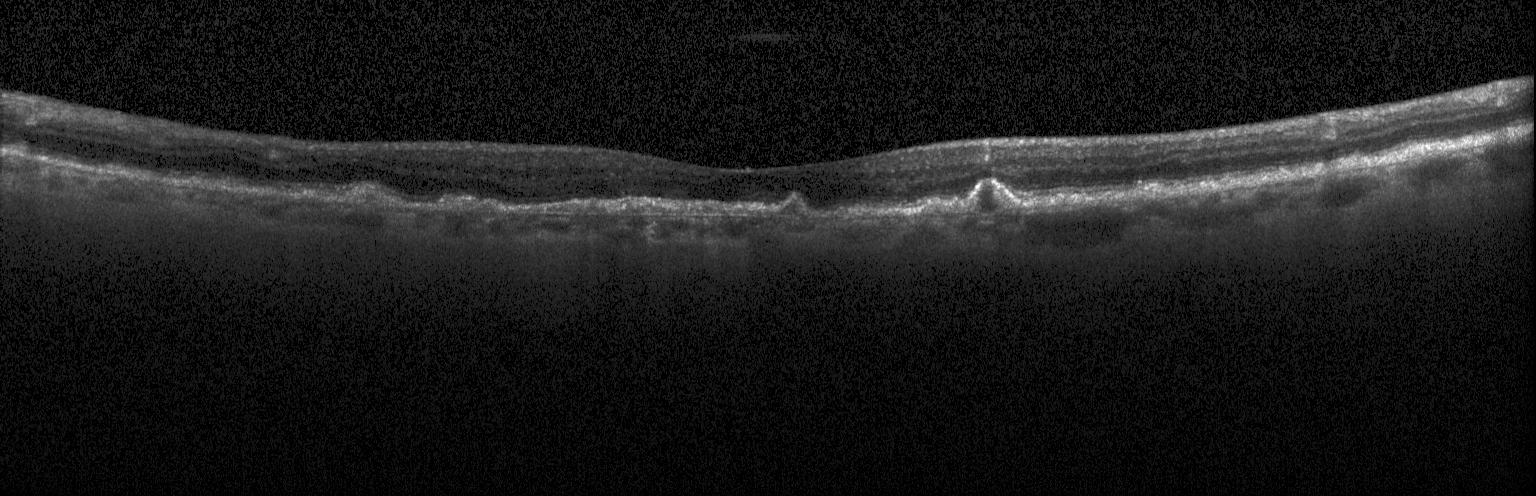 Dx: a choroidal neovascular membrane.